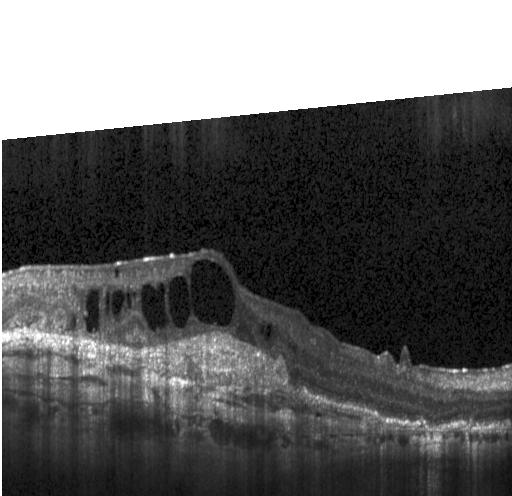
Macular OCT demonstrating a choroidal neovascular membrane.